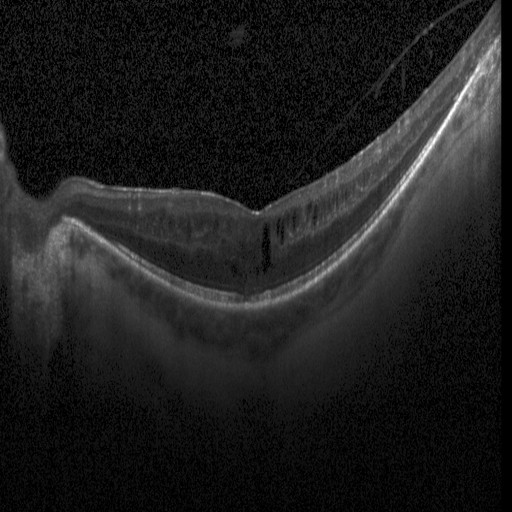

Optical coherence tomography scan, spectral-domain optical coherence tomography
This B-scan demonstrates DME.